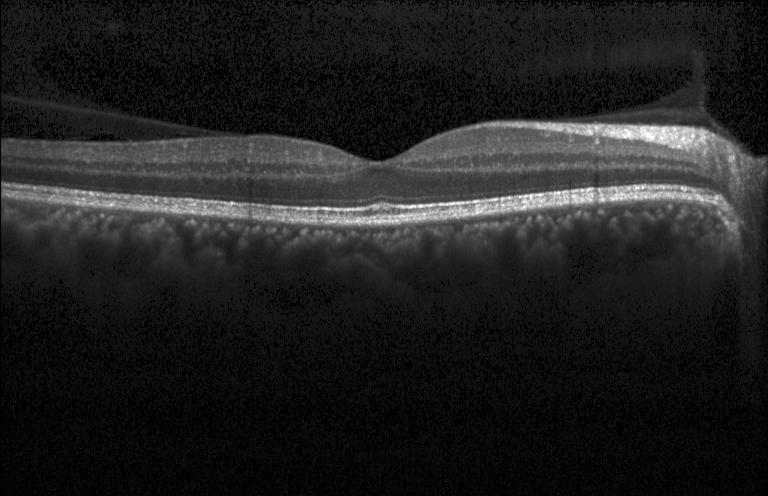 SD-OCT; fovea-centered; retinal OCT B-scan
Dx: no evidence of choroidal neovascularization, diabetic macular edema, or drusen.